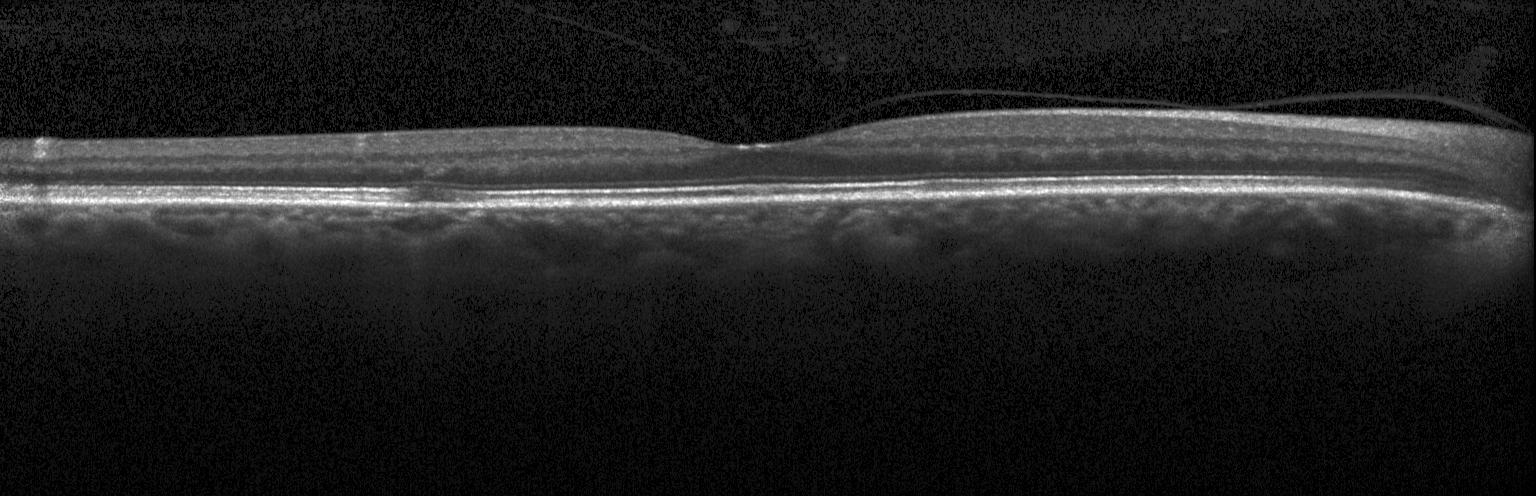 Dx: no evidence of CNV, DME, or drusen.